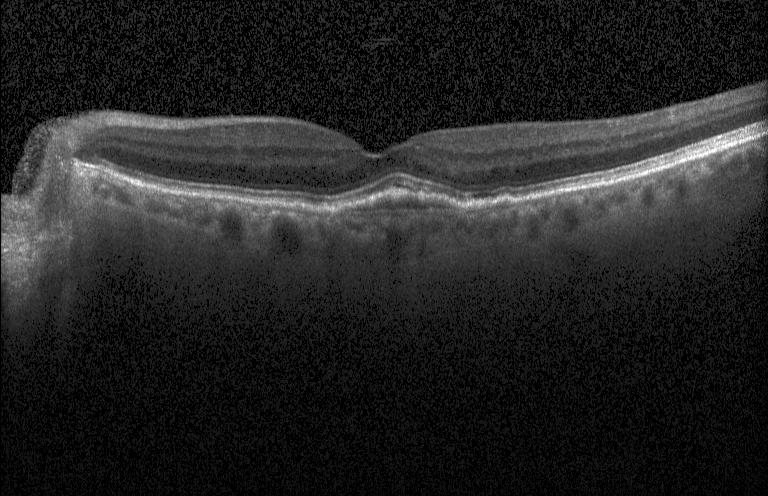 OCT scan showing a choroidal neovascular membrane.